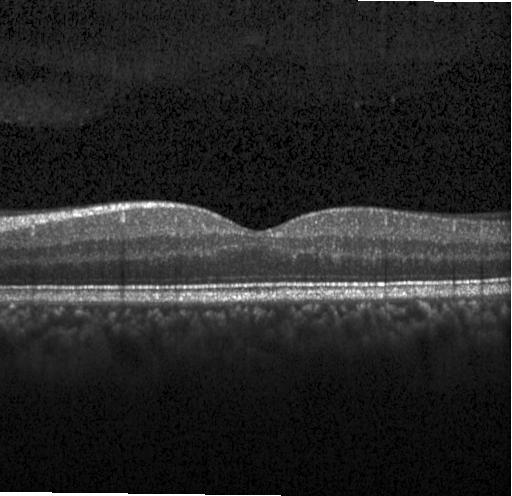
Instrument: Heidelberg Spectralis. Horizontal scan through the fovea. Retinal OCT cross-section. SD-OCT. The scan shows no evidence of choroidal neovascularization, diabetic macular edema, or drusen.